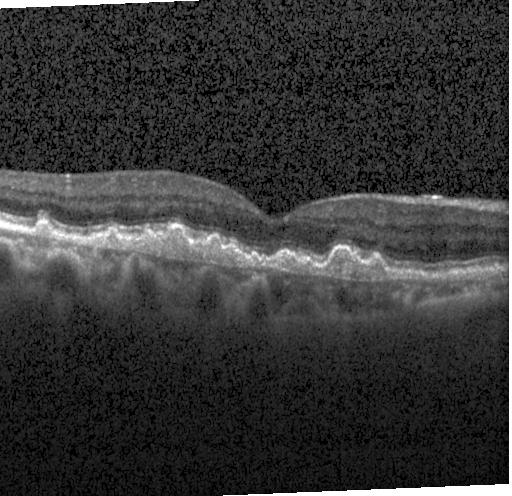
Spectral-domain OCT. Centered on the fovea. Optical coherence tomography B-scan — The scan shows choroidal neovascularization (CNV).